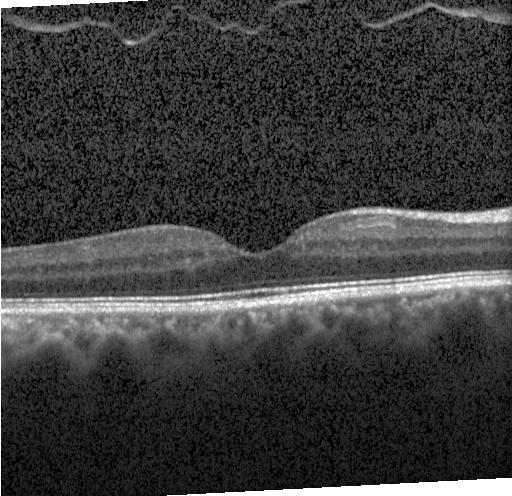
Spectral-domain OCT, optical coherence tomography B-scan
The scan shows no choroidal neovascularization, diabetic macular edema, or drusen.